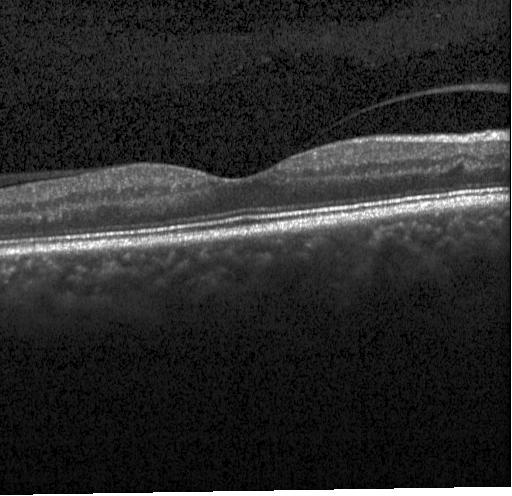
Retinal OCT cross-section showing no evidence of choroidal neovascularization, diabetic macular edema, or drusen.